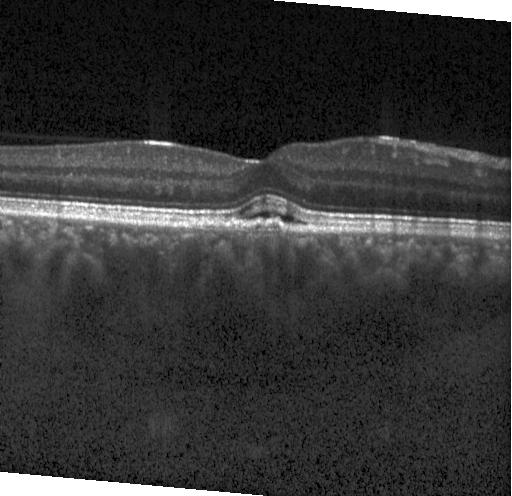 Through the macula. Heidelberg Spectralis. SD-OCT. Optical coherence tomography scan
Assessment: choroidal neovascularization (CNV).